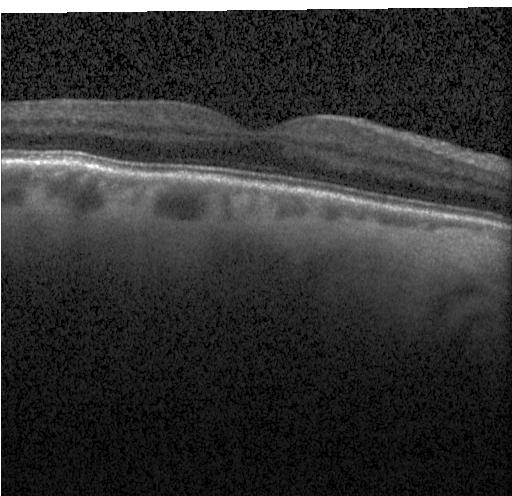 Retinal OCT cross-section. Macular scan
Impression: no CNV, DME, or drusen.